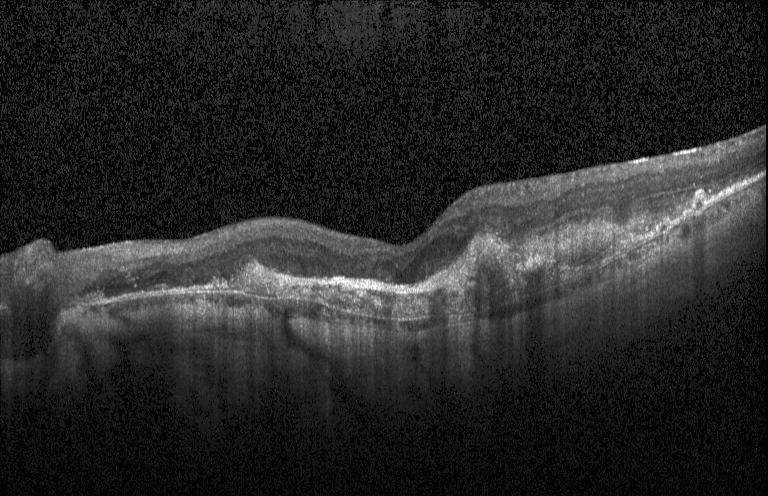
Retinal OCT cross-section. Through the macula. Spectral-domain optical coherence tomography.
Impression: CNV.